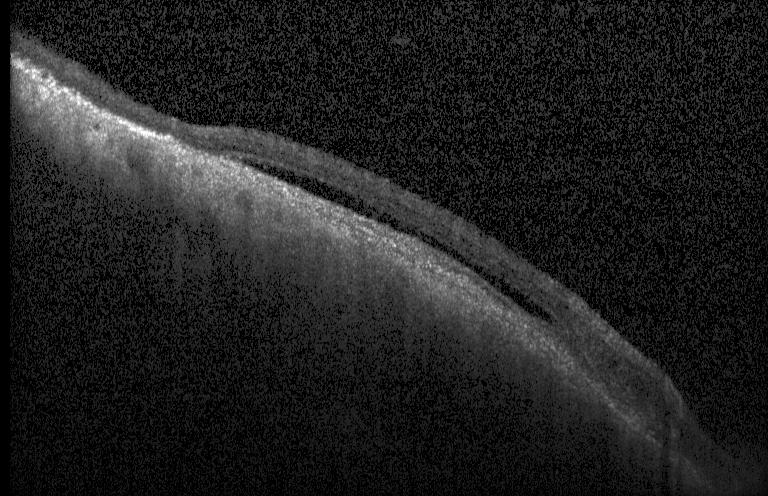 Heidelberg Spectralis; OCT B-scan; fovea-centered; spectral-domain optical coherence tomography. Diagnosis: choroidal neovascularization (CNV).